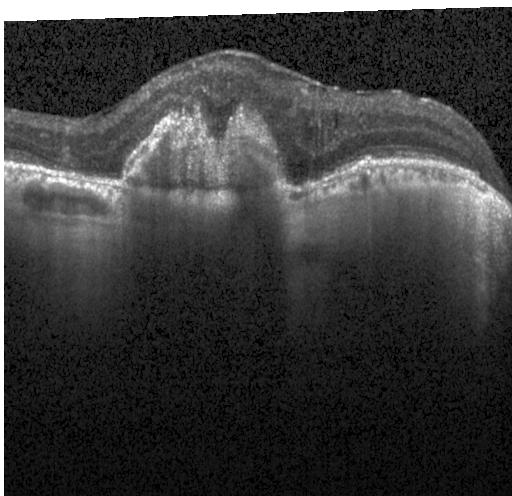
Finding: a choroidal neovascular membrane.